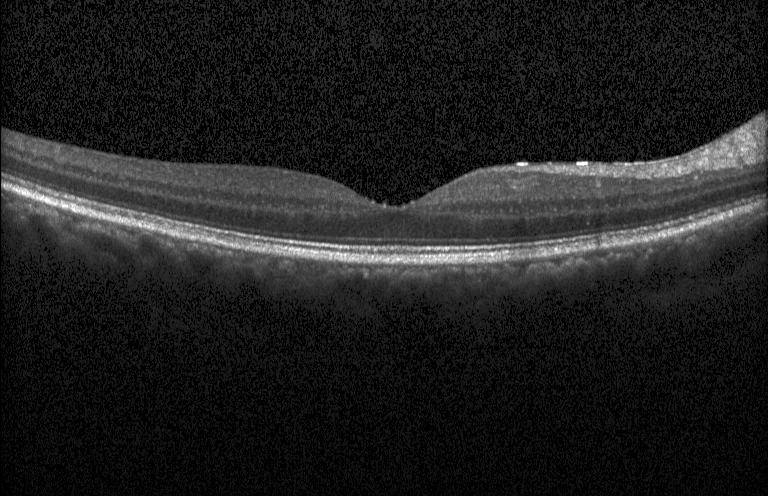 Dx: no CNV, DME, or drusen.